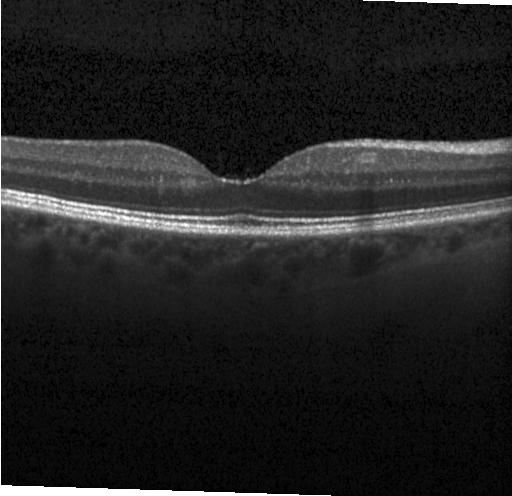 Retinal OCT B-scan · centered on the fovea · instrument: Heidelberg Spectralis · spectral-domain OCT. The scan shows neither choroidal neovascularization, diabetic macular edema, nor drusen.